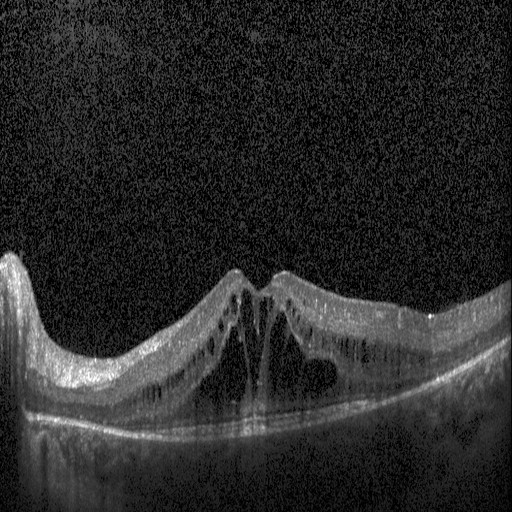
Macular OCT demonstrating DME.